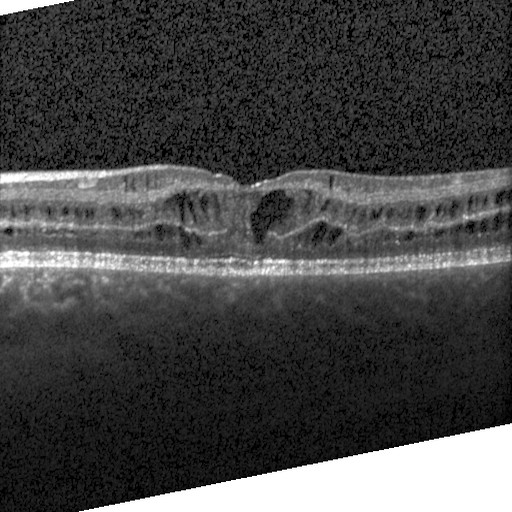
Retinal OCT cross-section showing diabetic macular edema (DME).